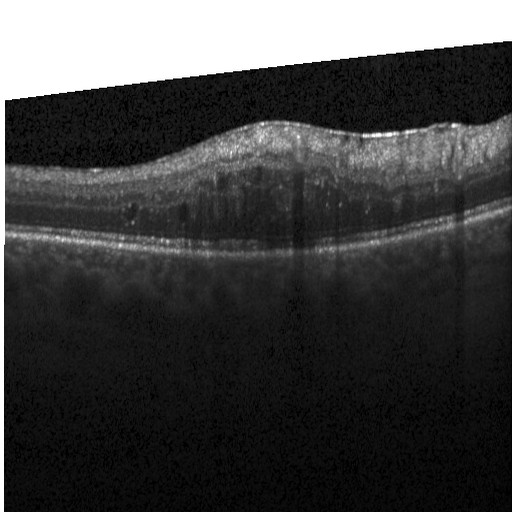

Retinal OCT cross-section
Finding: diabetic macular edema.